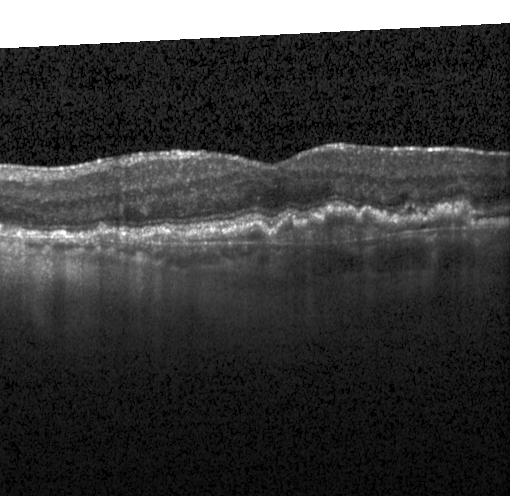
Assessment: CNV.